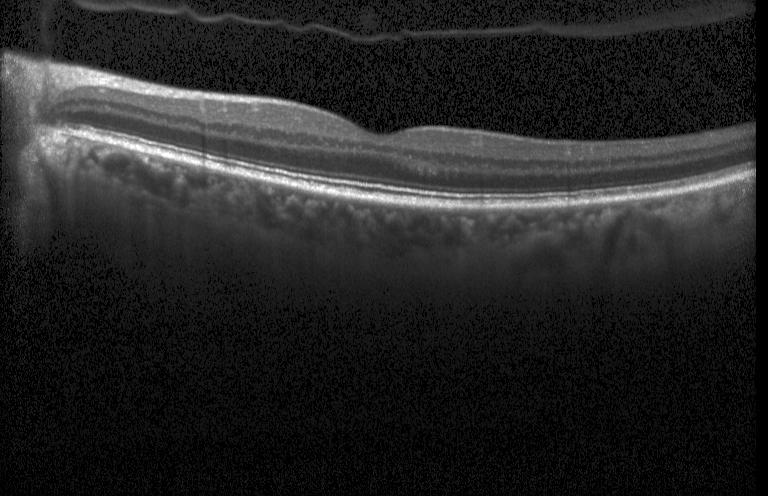 Finding: no choroidal neovascularization, no diabetic macular edema, and no drusen.